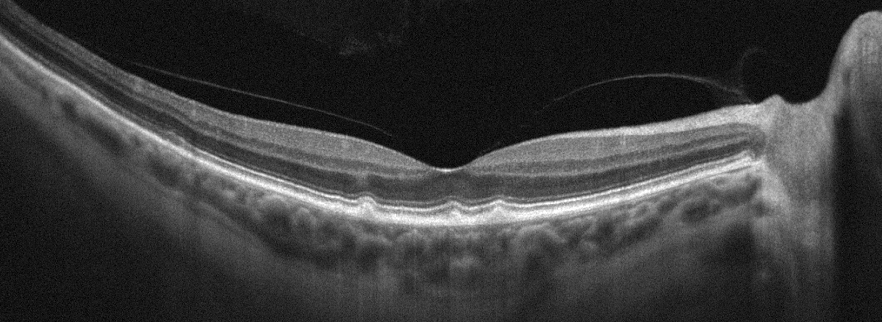 Impression: age-related macular degeneration (AMD).